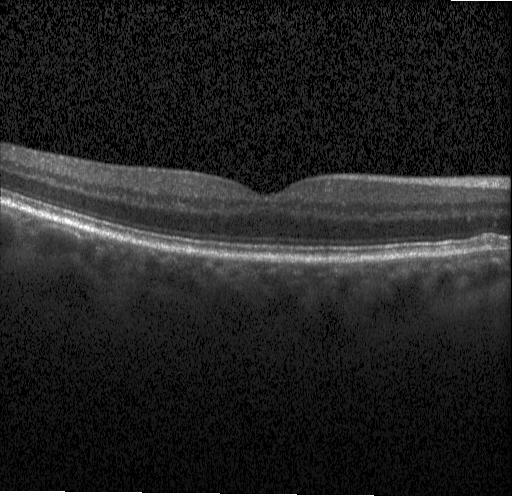
OCT line scan. SD-OCT. Heidelberg Spectralis — Finding: no evidence of CNV, DME, or drusen.